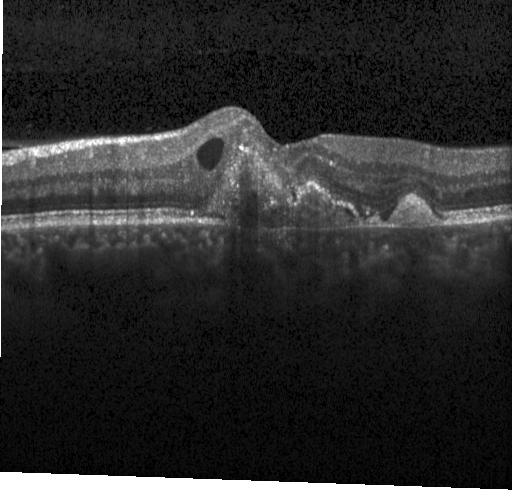
Instrument: Heidelberg Spectralis, SD-OCT, retinal OCT cross-section — Choroidal neovascularization.